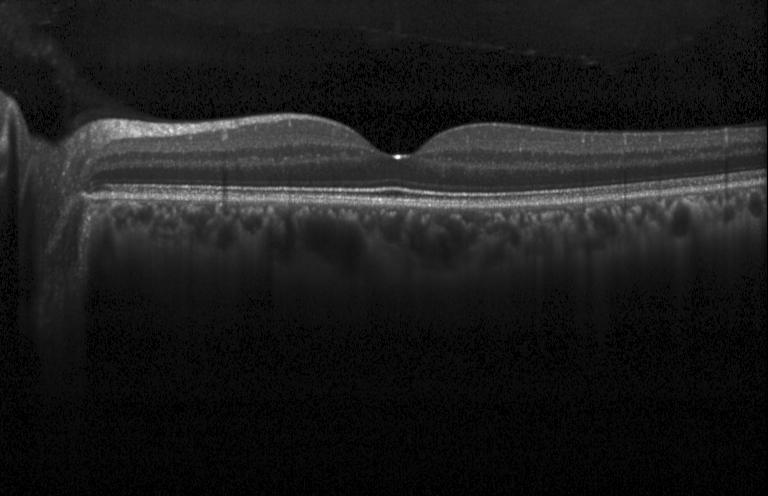 Retinal OCT cross-section.
Assessment: no choroidal neovascularization, no diabetic macular edema, and no drusen.